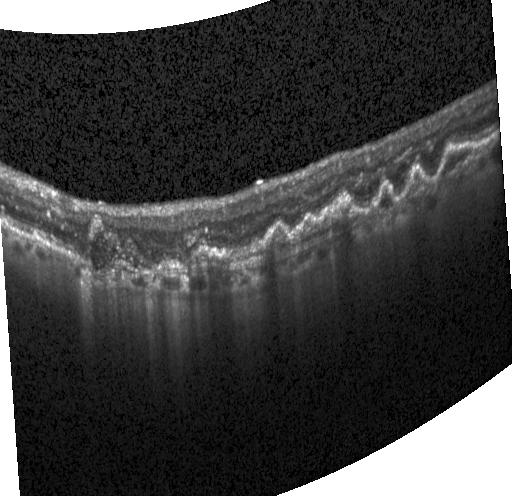
Centered on the fovea, OCT B-scan, instrument: Heidelberg Spectralis. CNV.